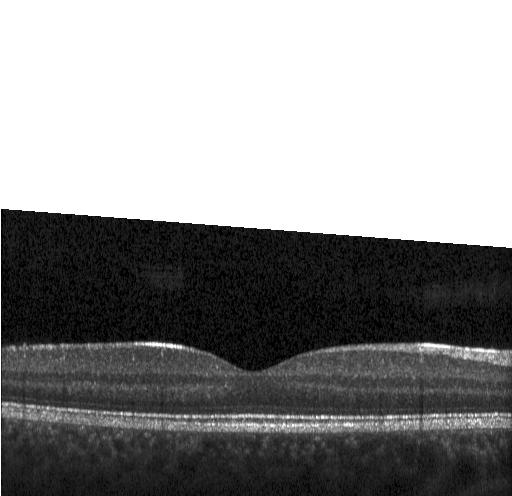 Spectral-domain optical coherence tomography · OCT B-scan · instrument: Heidelberg Spectralis. Assessment: no evidence of choroidal neovascularization, diabetic macular edema, or drusen.